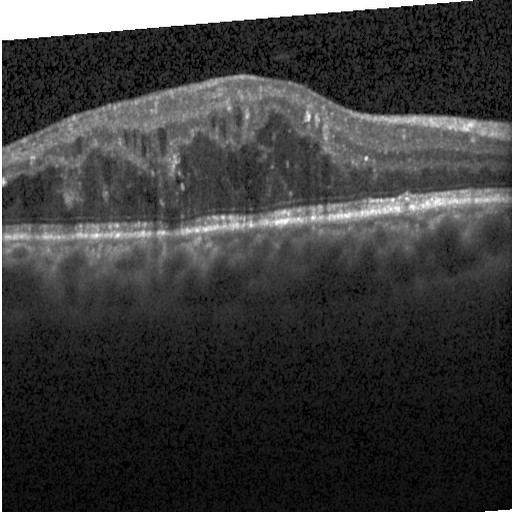

Acquired on a Heidelberg Spectralis. SD-OCT. Fovea-centered. Optical coherence tomography B-scan.
This B-scan demonstrates DME.